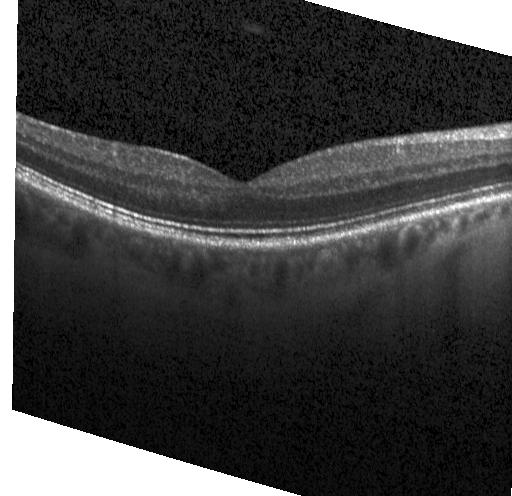 Instrument: Heidelberg Spectralis, SD-OCT, optical coherence tomography B-scan. Assessment: no choroidal neovascularization, diabetic macular edema, or drusen.